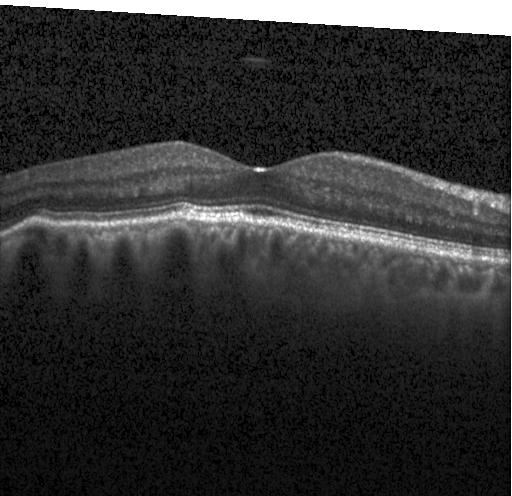
Spectral-domain optical coherence tomography. Centered on the fovea. Heidelberg Spectralis OCT system. Retinal OCT cross-section.
Assessment: no evidence of choroidal neovascularization, diabetic macular edema, or drusen.